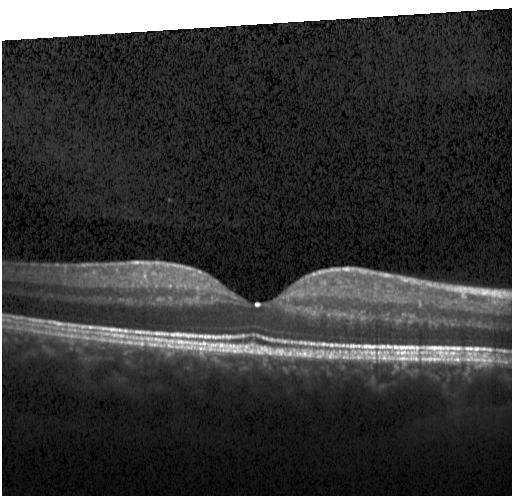 Finding: no choroidal neovascularization, no diabetic macular edema, and no drusen.